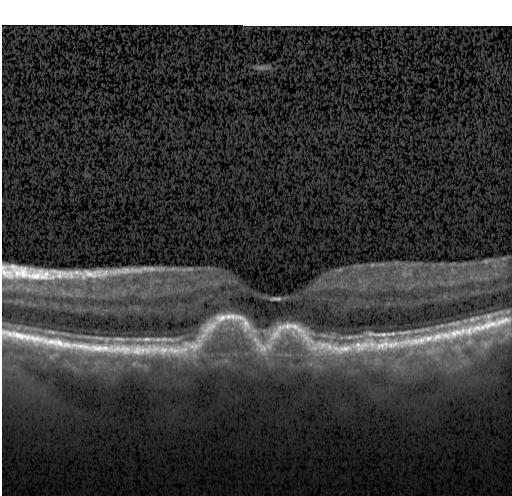

Heidelberg Spectralis; SD-OCT; optical coherence tomography scan.
Impression: drusen.